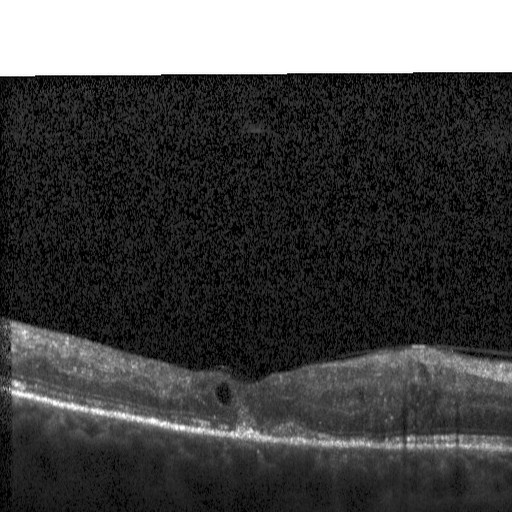 Assessment: DME.